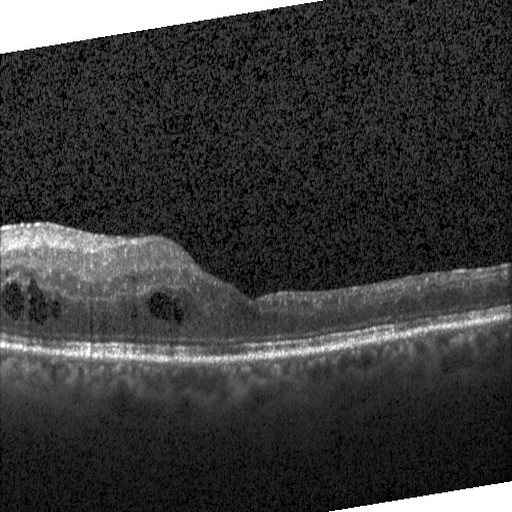
Retinal OCT B-scan, centered on the fovea. Impression: diabetic macular edema (DME).